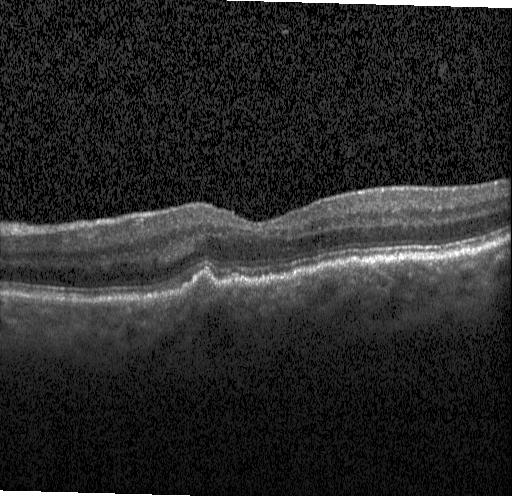

Heidelberg Spectralis · OCT B-scan · spectral-domain optical coherence tomography — This B-scan demonstrates drusen.